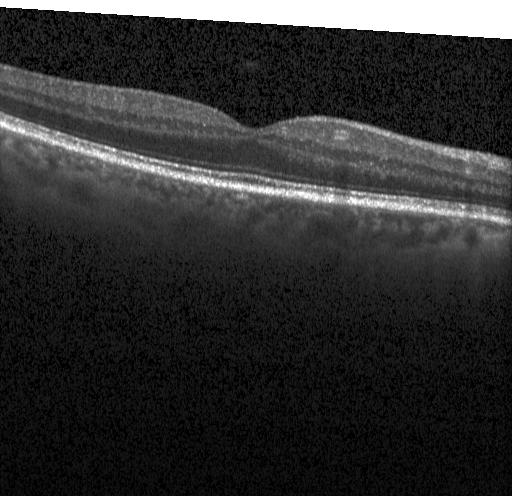
SD-OCT · horizontal scan through the fovea · optical coherence tomography B-scan · acquired on a Heidelberg Spectralis.
This B-scan demonstrates no choroidal neovascularization, diabetic macular edema, or drusen.